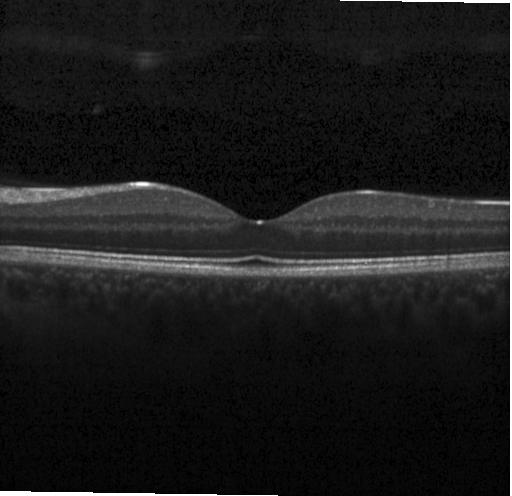
Diagnosis: no choroidal neovascularization, no diabetic macular edema, and no drusen.